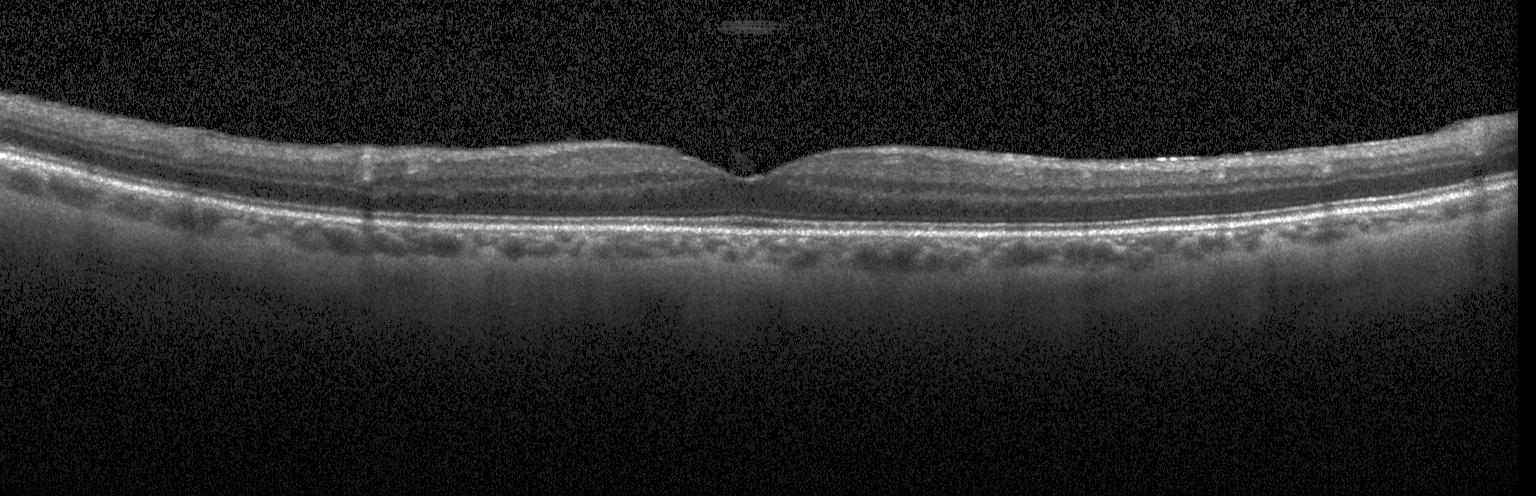

Acquired on a Heidelberg Spectralis. Retinal OCT cross-section. SD-OCT. Centered on the fovea
Diagnosis: neither choroidal neovascularization, diabetic macular edema, nor drusen.